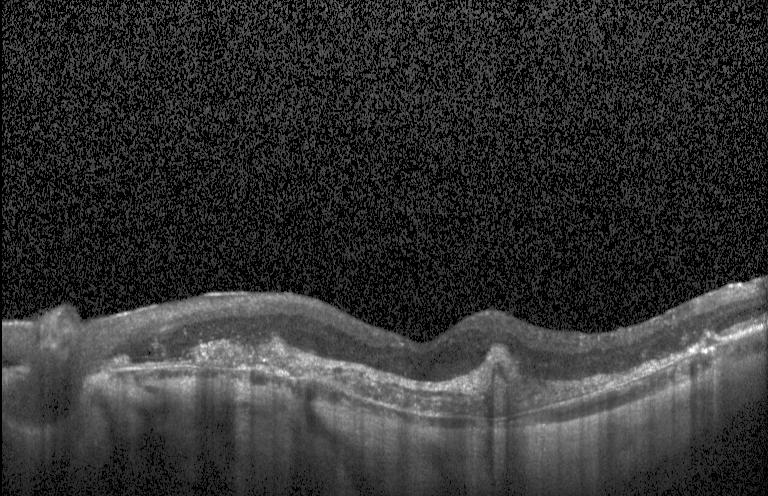

Dx: choroidal neovascularization (CNV).